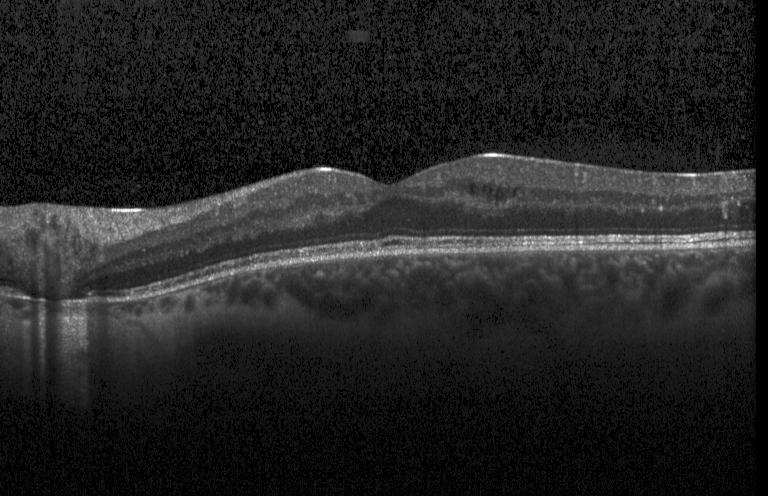

OCT scan showing DME.